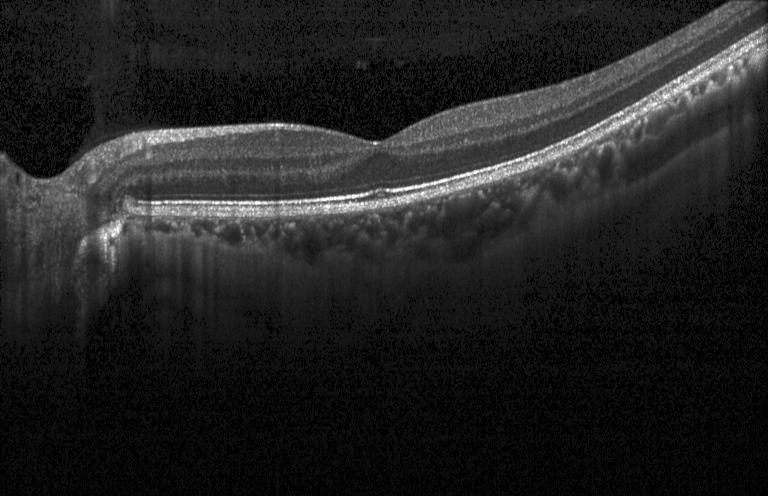
OCT B-scan showing neither CNV, DME, nor drusen.